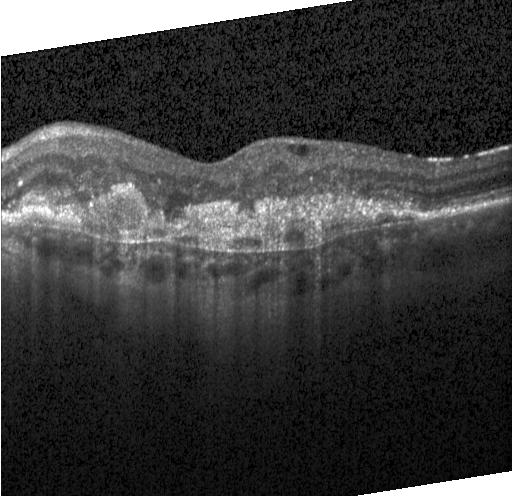 Diagnosis: a choroidal neovascular membrane.